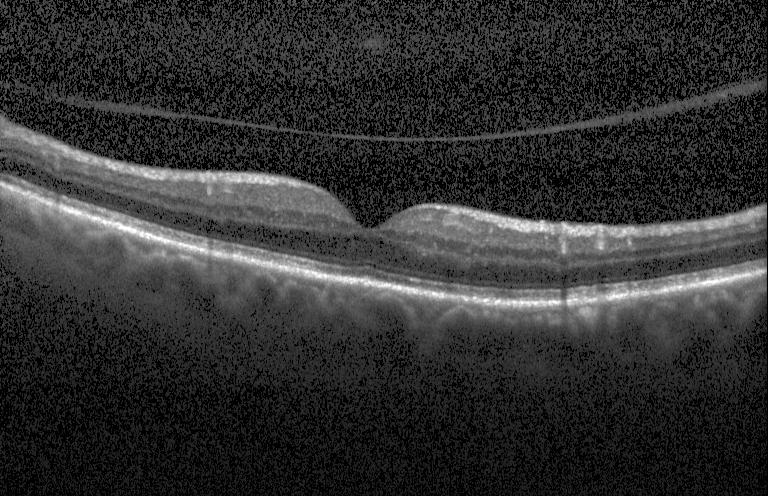 Optical coherence tomography scan
This B-scan demonstrates no choroidal neovascularization, no diabetic macular edema, and no drusen.